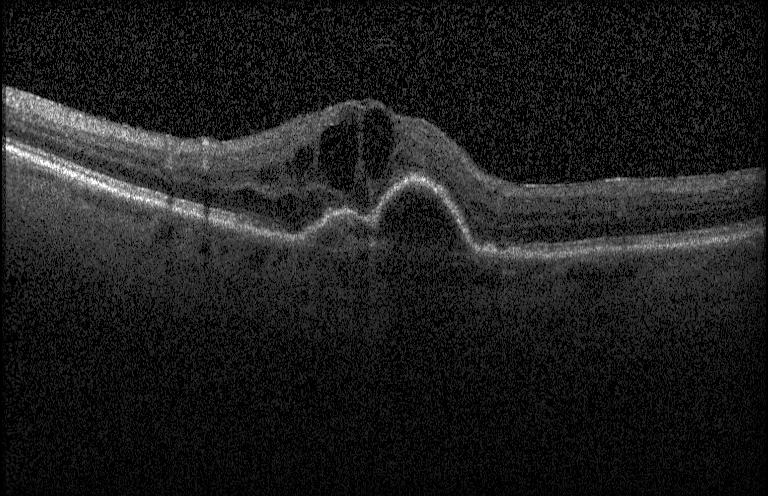

Fovea-centered, SD-OCT, OCT B-scan, Heidelberg Spectralis — Assessment: a choroidal neovascular membrane.